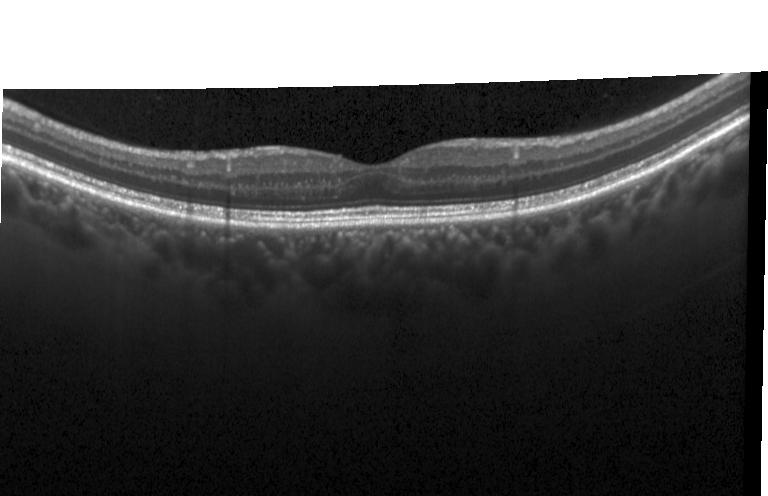
Dx: neither choroidal neovascularization, diabetic macular edema, nor drusen.